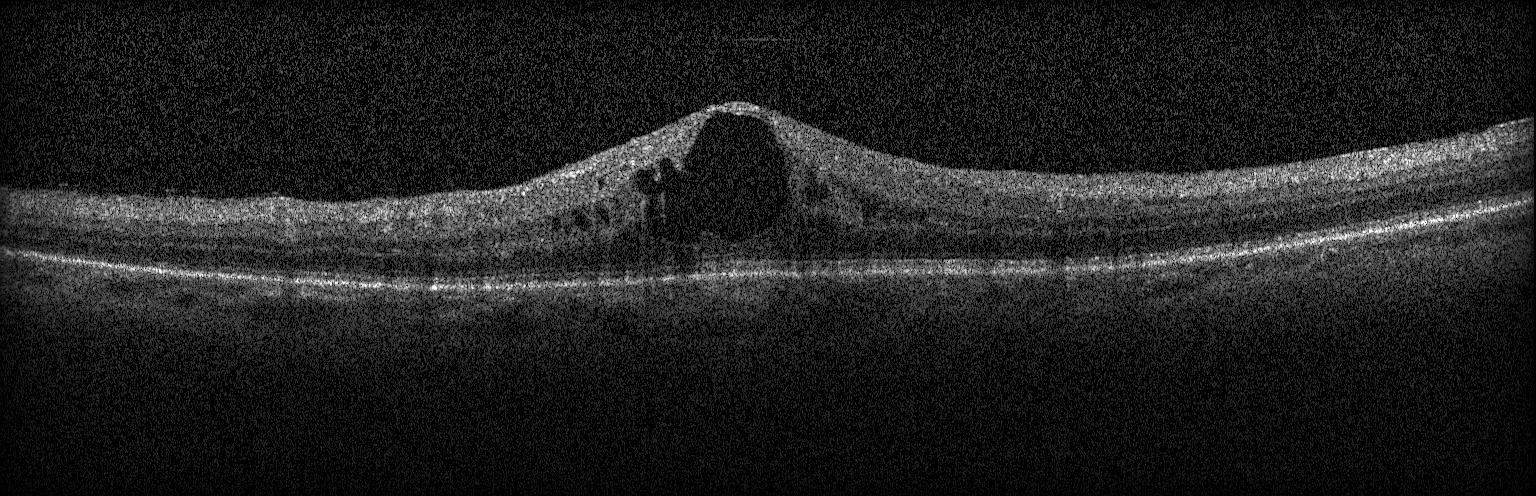

Optical coherence tomography B-scan; Heidelberg Spectralis; horizontal scan through the fovea
Macular OCT: diabetic macular edema.